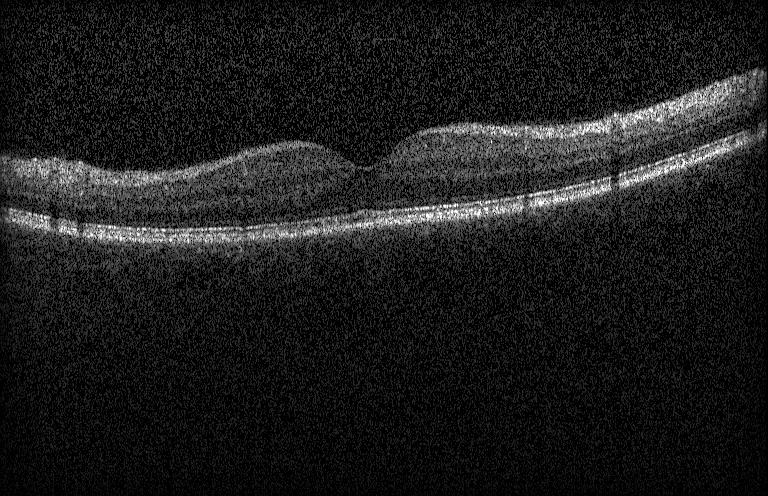
Assessment: no CNV, no DME, and no drusen.